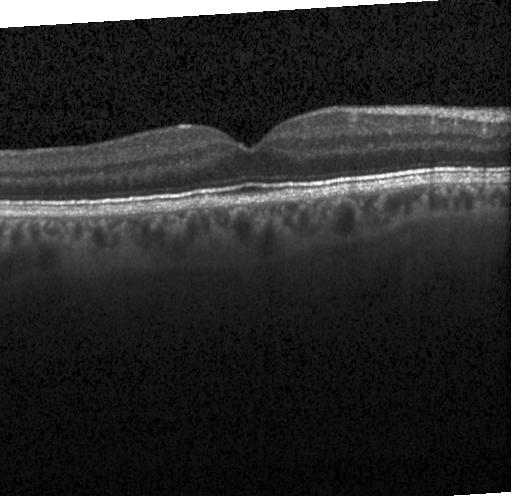

Retinal OCT cross-section. Instrument: Heidelberg Spectralis.
No CNV, no DME, and no drusen.